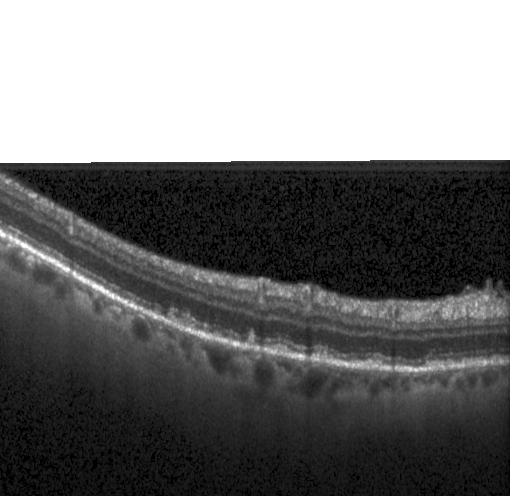
OCT B-scan · SD-OCT. Diagnosis: drusen.